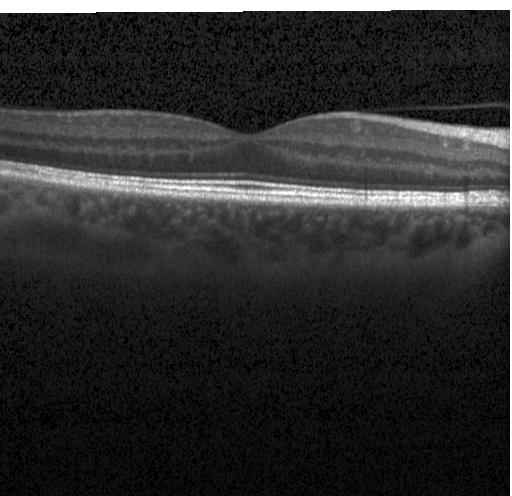
OCT finding: no evidence of choroidal neovascularization, diabetic macular edema, or drusen.